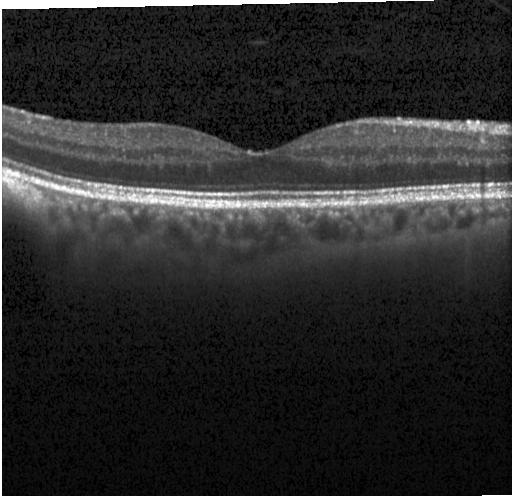
OCT line scan. Assessment: no choroidal neovascularization, no diabetic macular edema, and no drusen.